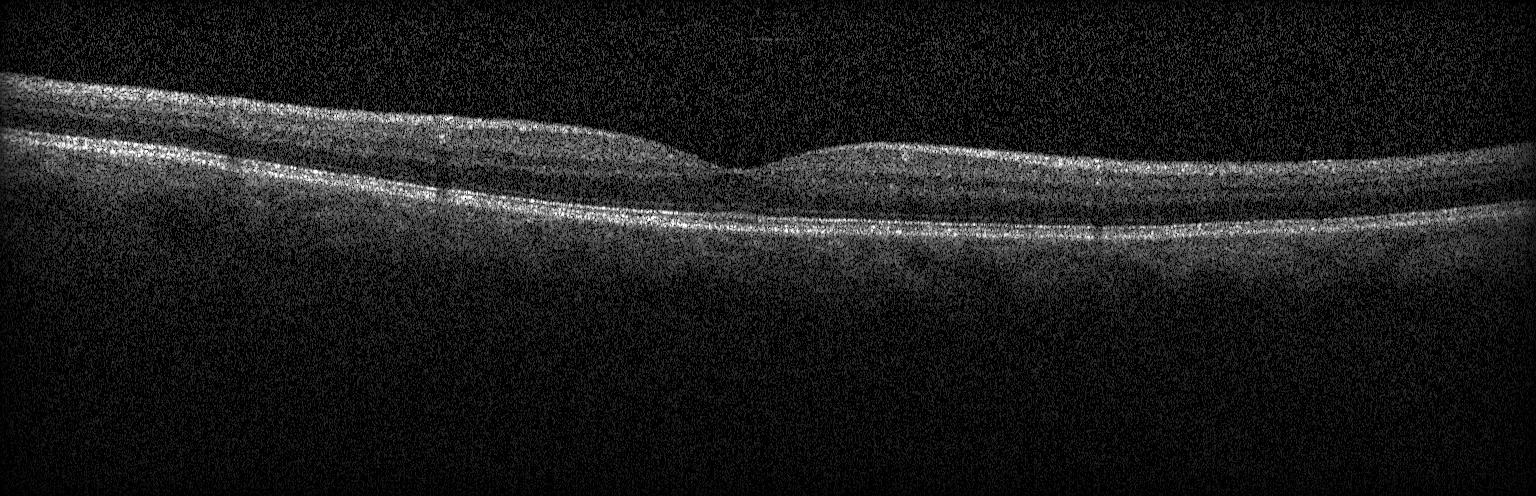 Heidelberg Spectralis. OCT B-scan. Horizontal scan through the fovea. Spectral-domain optical coherence tomography — Diagnosis: neither choroidal neovascularization, diabetic macular edema, nor drusen.